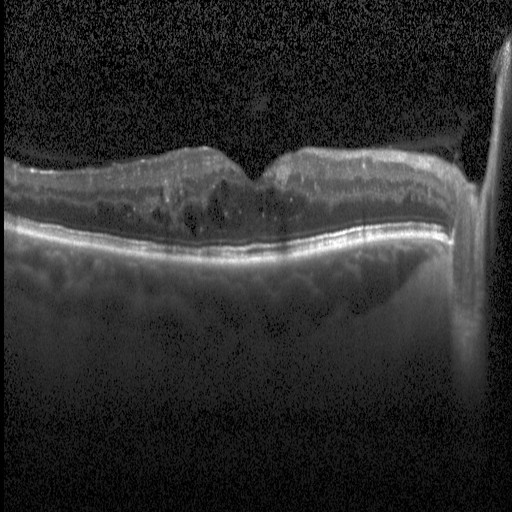 Optical coherence tomography B-scan. Heidelberg Spectralis. Horizontal scan through the fovea. DME.